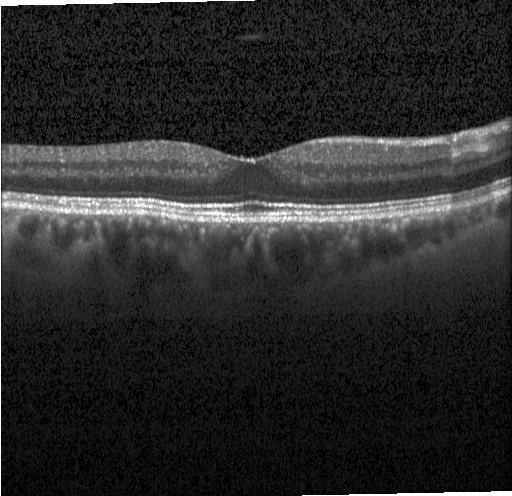

Instrument: Heidelberg Spectralis. OCT line scan. Spectral-domain OCT. Centered on the fovea — Finding: no choroidal neovascularization, no diabetic macular edema, and no drusen.